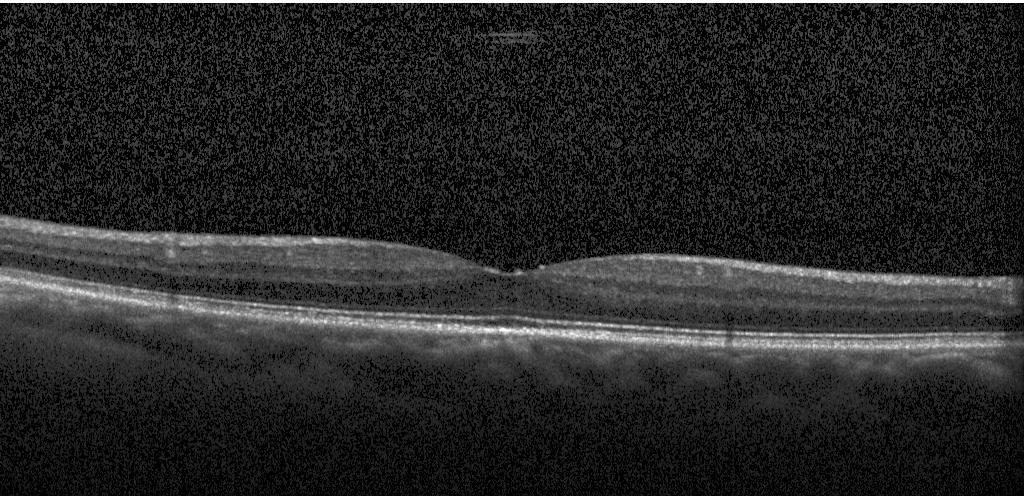

Retinal OCT cross-section showing neither choroidal neovascularization, diabetic macular edema, nor drusen.